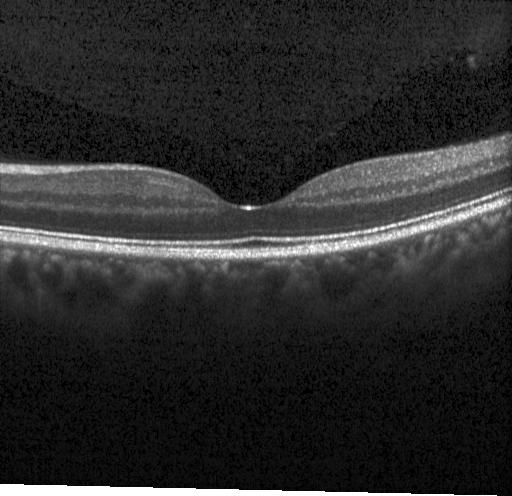

Diagnosis: neither choroidal neovascularization, diabetic macular edema, nor drusen.